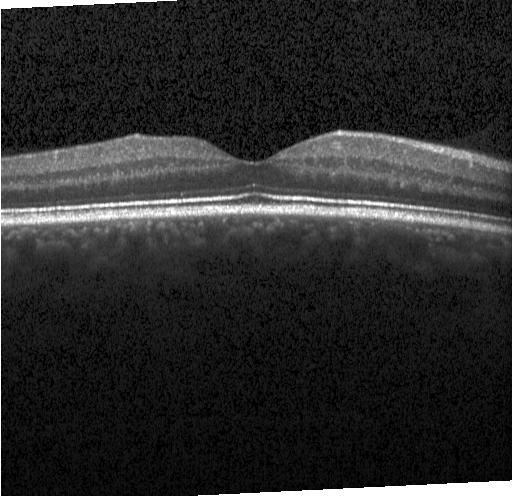

Centered on the fovea. Retinal OCT cross-section — The scan shows neither choroidal neovascularization, diabetic macular edema, nor drusen.